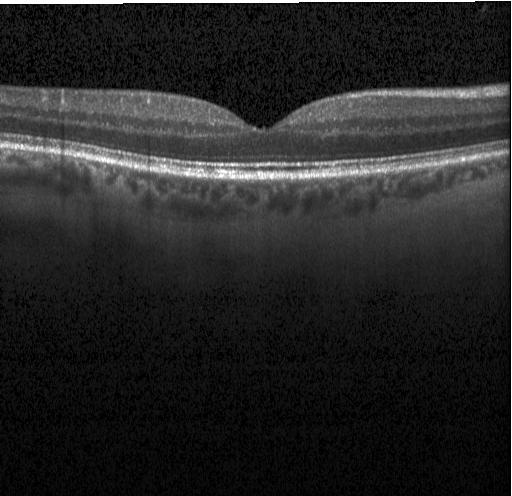
Spectral-domain OCT. Centered on the fovea. Retinal OCT cross-section.
Impression: no choroidal neovascularization, diabetic macular edema, or drusen.